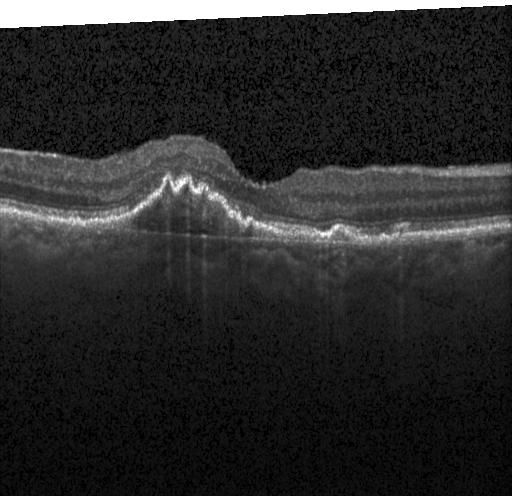 Retinal OCT cross-section · through the macula
Impression: choroidal neovascularization (CNV).